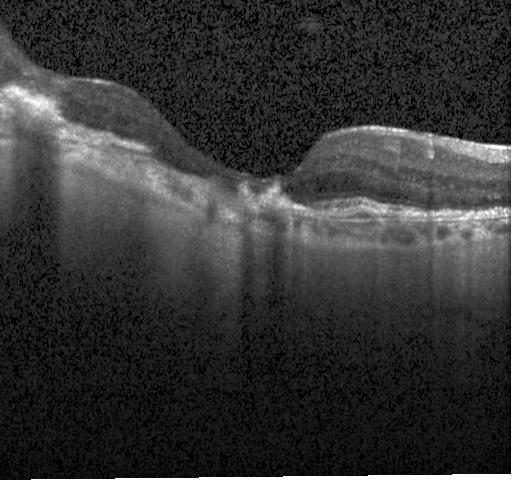 Spectral-domain OCT B-scan: a choroidal neovascular membrane.